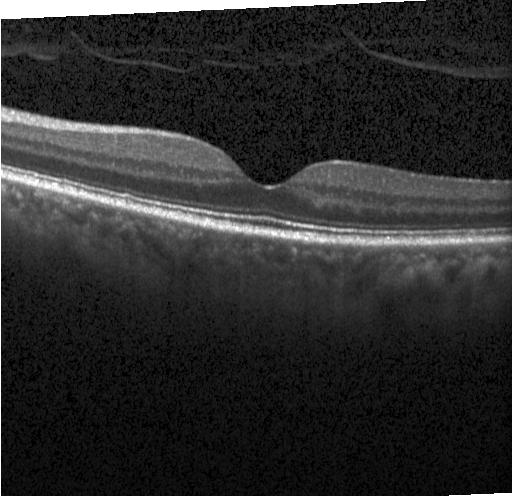 Heidelberg Spectralis, macular scan, OCT line scan, SD-OCT — The scan shows neither choroidal neovascularization, diabetic macular edema, nor drusen.